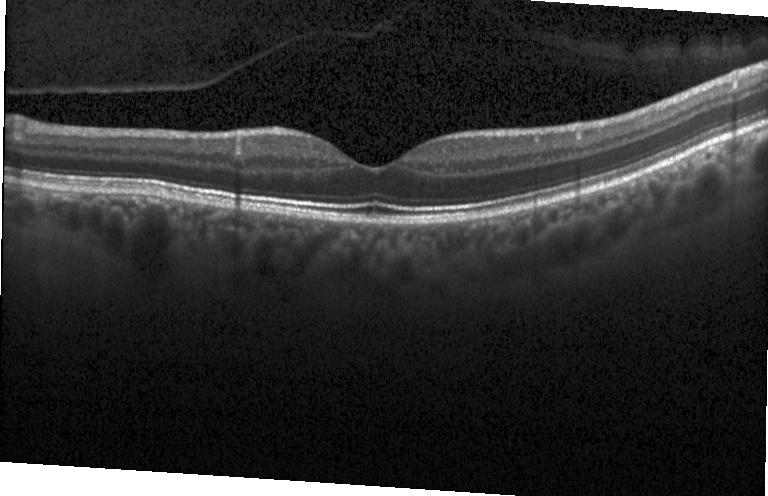

Retinal OCT B-scan, acquired on a Heidelberg Spectralis, SD-OCT, through the macula — Diagnosis: no choroidal neovascularization, no diabetic macular edema, and no drusen.